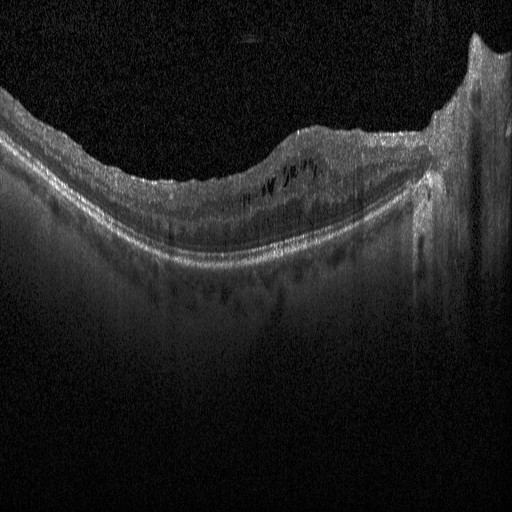
Spectral-domain optical coherence tomography; OCT B-scan; centered on the fovea — This B-scan demonstrates DME.